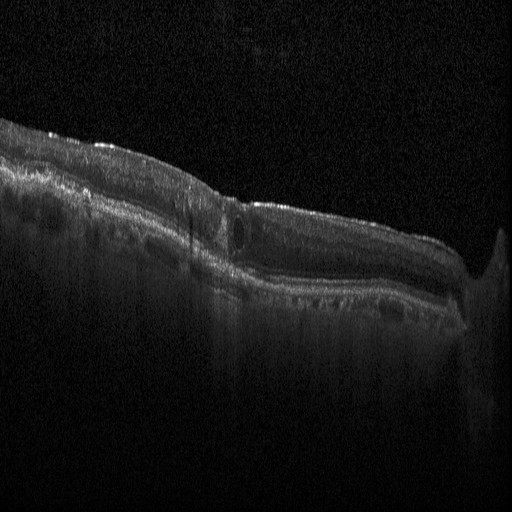
Acquired on a Heidelberg Spectralis. OCT line scan — Finding: diabetic macular edema (DME).